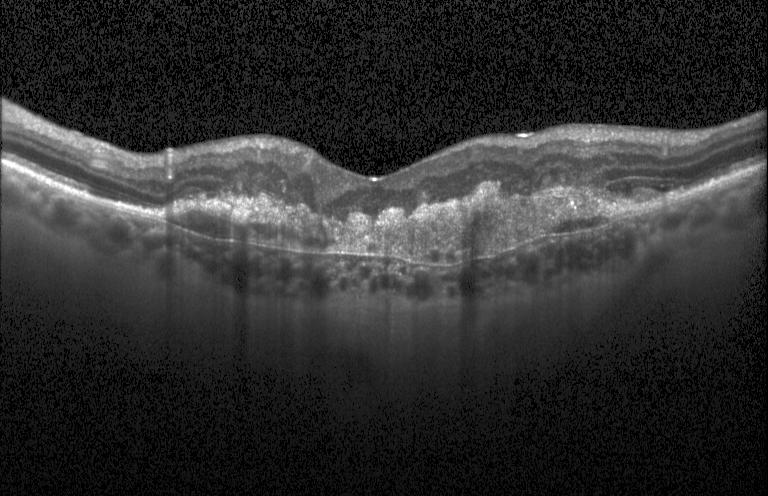

Instrument: Heidelberg Spectralis. Spectral-domain OCT. Macular scan. Retinal OCT B-scan. Impression: choroidal neovascularization (CNV).